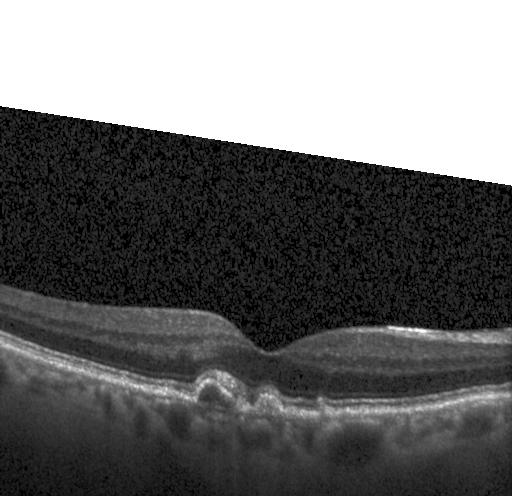

Acquired on a Heidelberg Spectralis · centered on the fovea · spectral-domain optical coherence tomography · retinal OCT cross-section
A choroidal neovascular membrane.